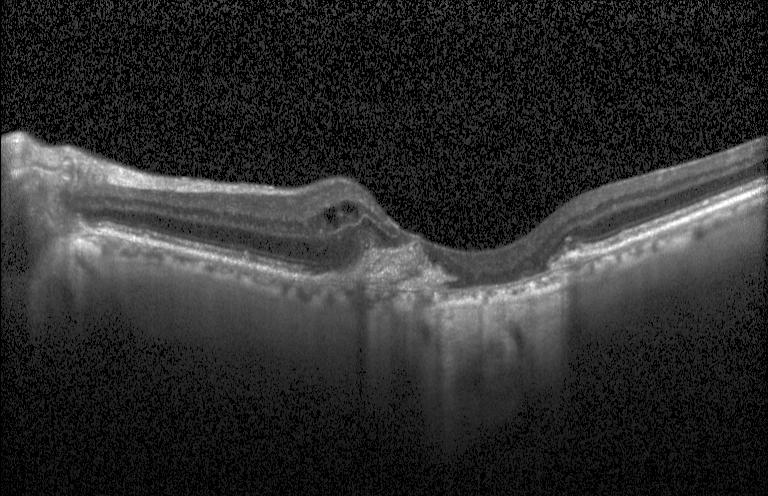
A choroidal neovascular membrane.